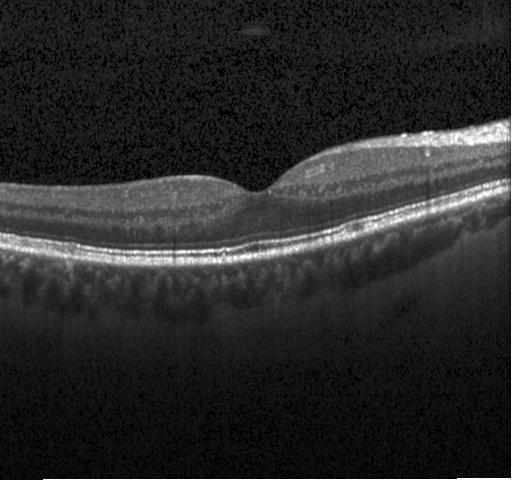
Assessment: no choroidal neovascularization, diabetic macular edema, or drusen.